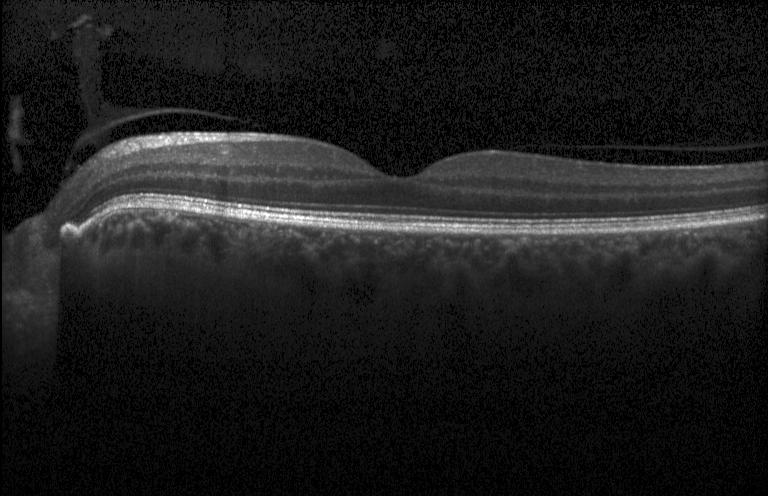 Optical coherence tomography B-scan
Impression: no choroidal neovascularization, diabetic macular edema, or drusen.